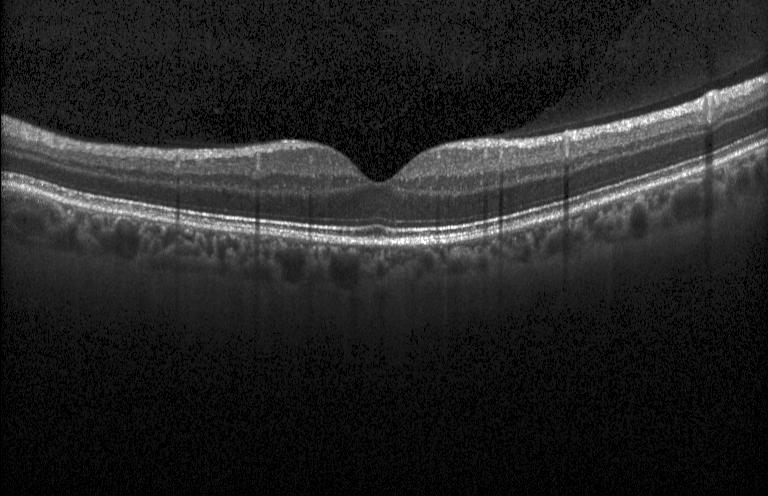

Instrument: Heidelberg Spectralis · optical coherence tomography scan. Dx: no evidence of choroidal neovascularization, diabetic macular edema, or drusen.